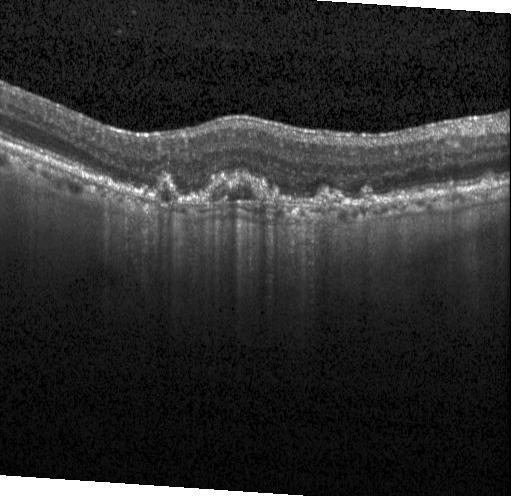
Retinal OCT cross-section
Diagnosis: a choroidal neovascular membrane.